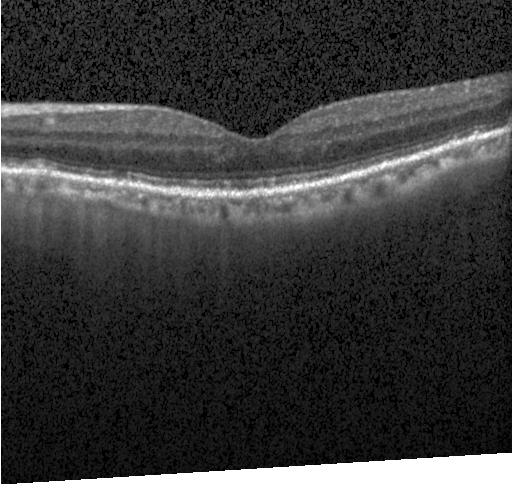 Optical coherence tomography scan — Assessment: no choroidal neovascularization, diabetic macular edema, or drusen.